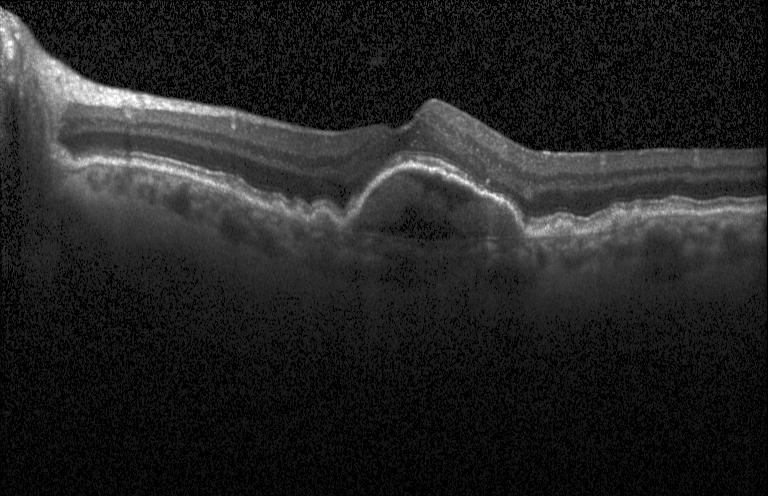 Retinal OCT cross-section; Heidelberg Spectralis.
Finding: sub-RPE drusenoid deposits.